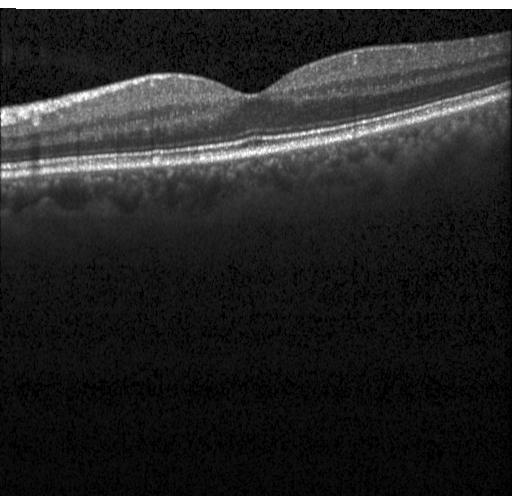
Spectral-domain optical coherence tomography. Horizontal scan through the fovea. Acquired on a Heidelberg Spectralis. Retinal OCT B-scan. Neither choroidal neovascularization, diabetic macular edema, nor drusen.